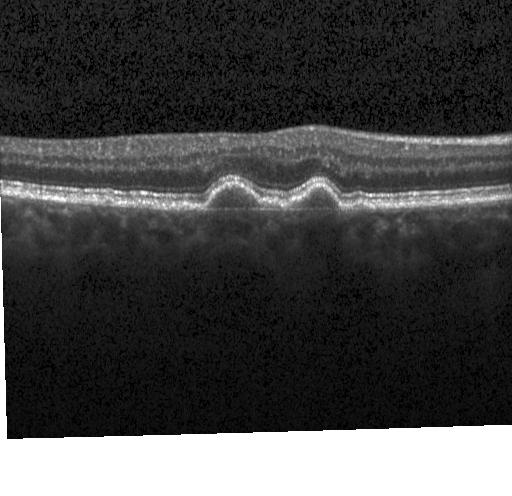

Assessment: drusen.